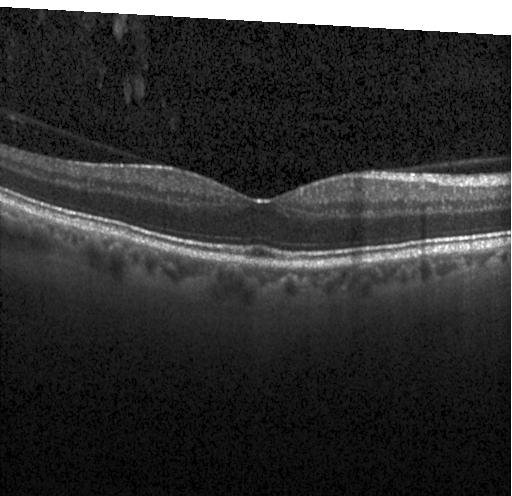

Instrument: Heidelberg Spectralis; retinal OCT cross-section. No CNV, no DME, and no drusen.